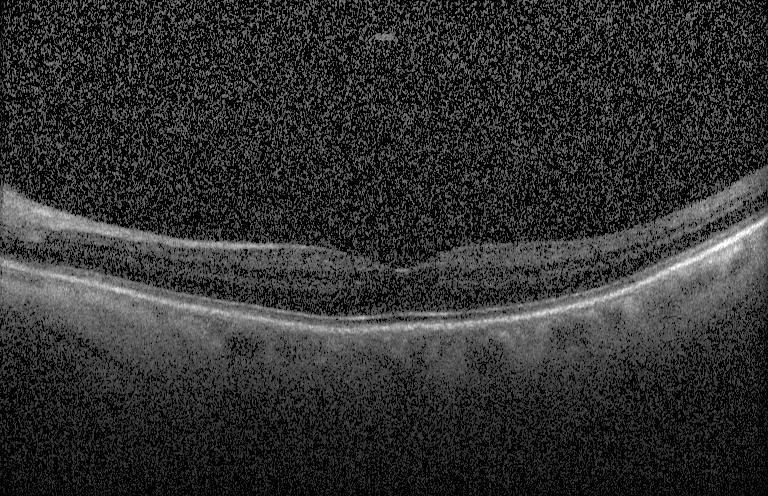
OCT B-scan.
OCT finding: no evidence of choroidal neovascularization, diabetic macular edema, or drusen.